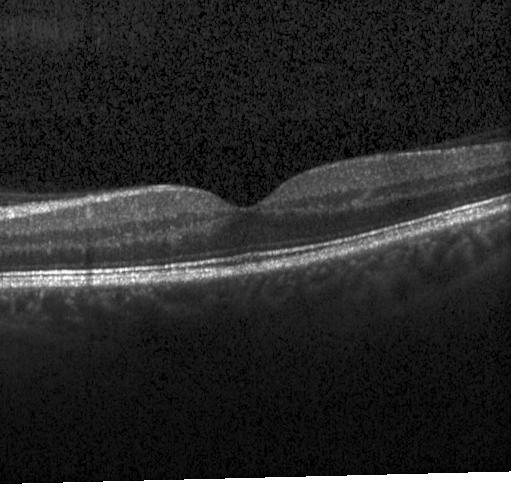

OCT B-scan — No choroidal neovascularization, diabetic macular edema, or drusen.